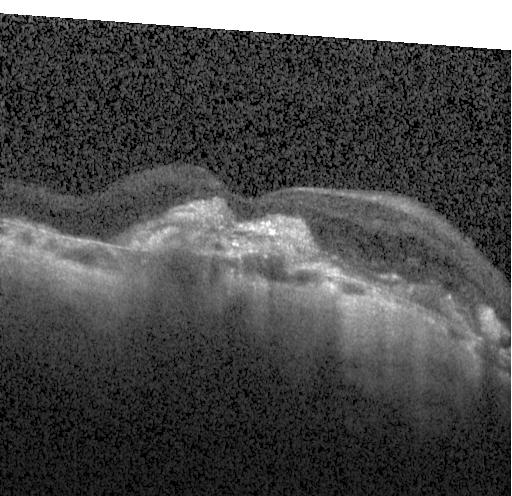

Finding: CNV.